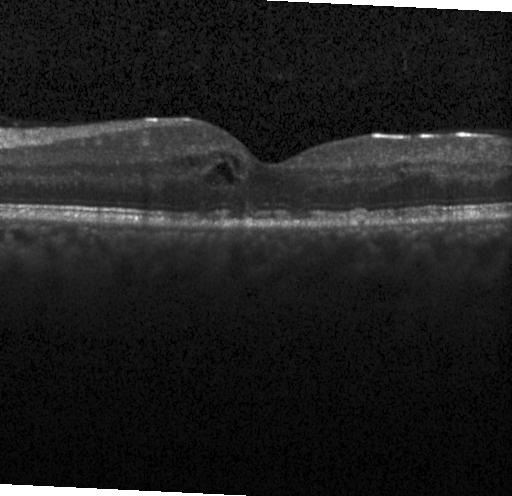 Through the macula, retinal OCT cross-section — This B-scan demonstrates DME.